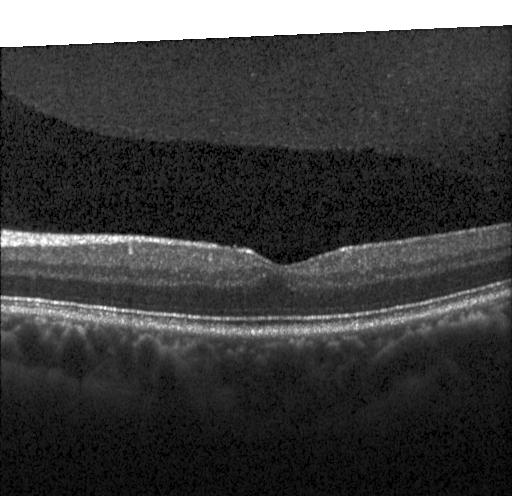

Finding: no CNV, DME, or drusen.